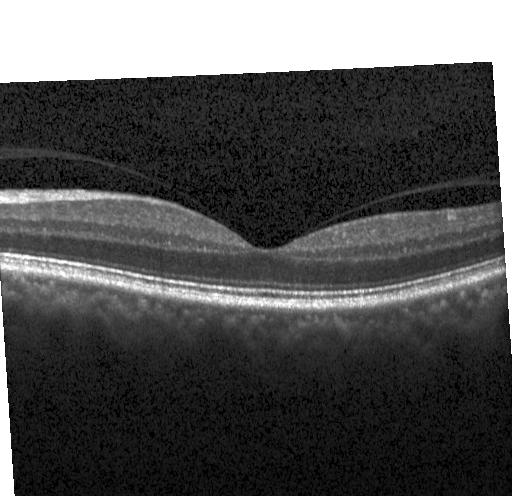
Assessment: no CNV, DME, or drusen.